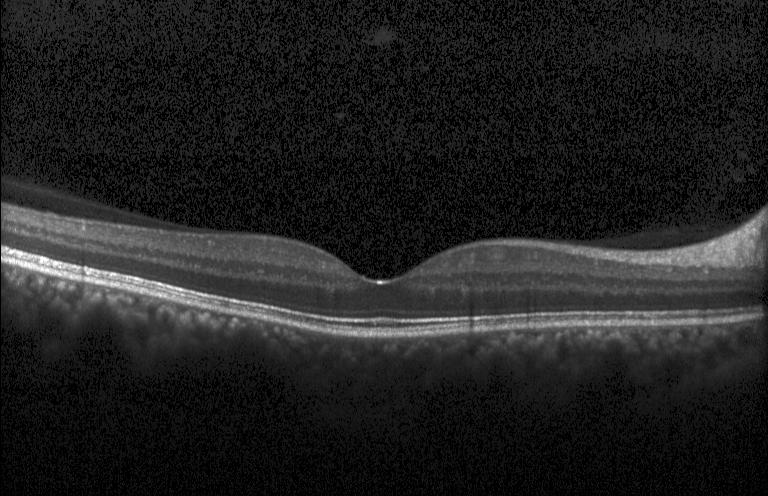
OCT B-scan, spectral-domain OCT. Impression: no choroidal neovascularization, no diabetic macular edema, and no drusen.